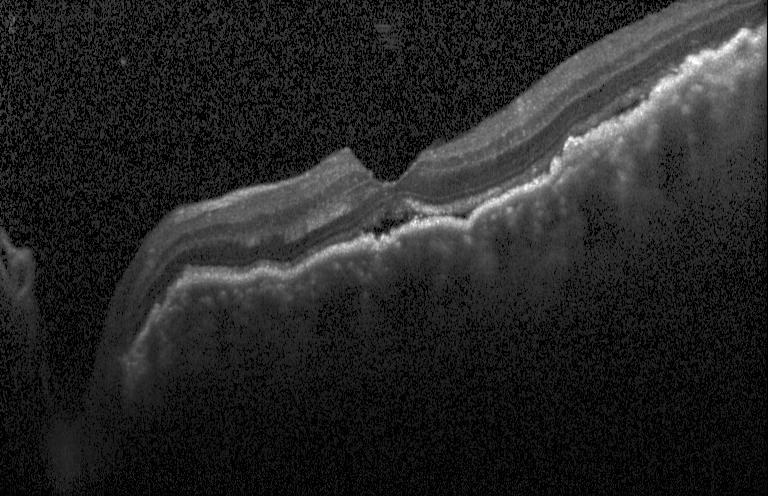 Impression: CNV.